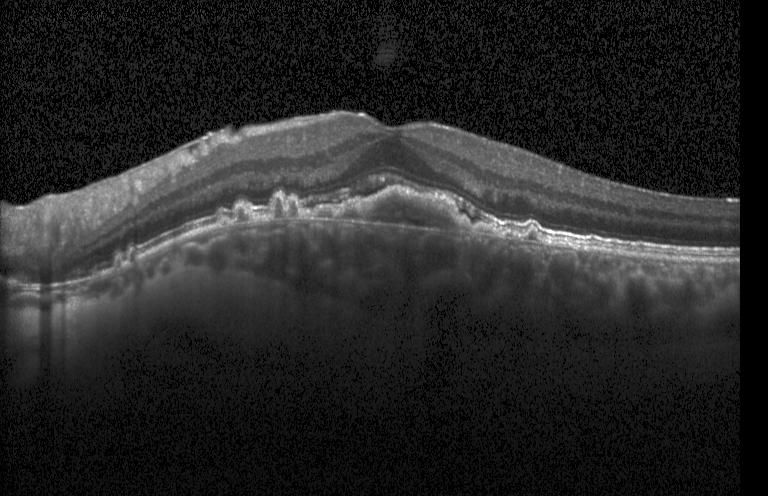 OCT B-scan · fovea-centered — Assessment: CNV.